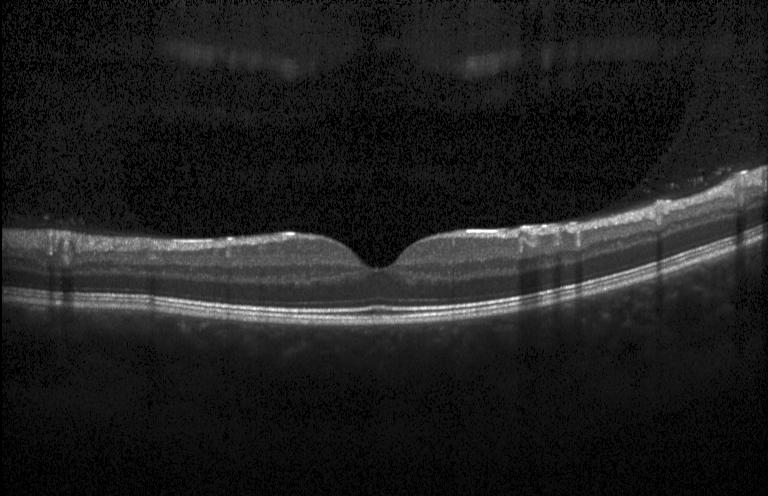

Retinal OCT B-scan. This B-scan demonstrates neither choroidal neovascularization, diabetic macular edema, nor drusen.